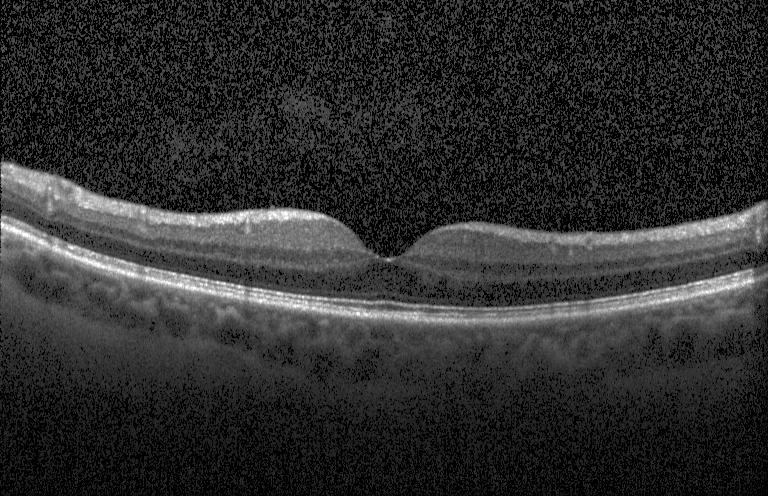

Acquired on a Heidelberg Spectralis · retinal OCT cross-section. Finding: no choroidal neovascularization, diabetic macular edema, or drusen.